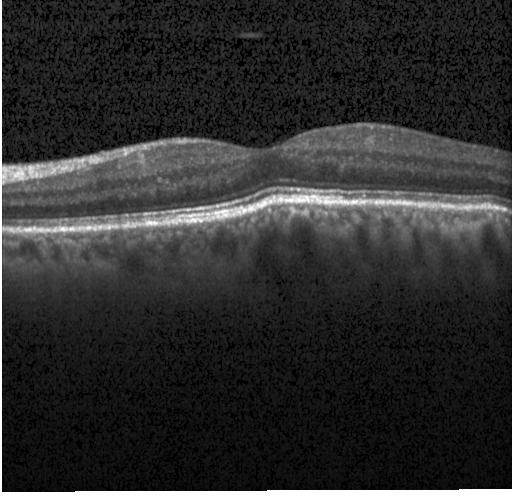

Horizontal scan through the fovea; retinal OCT B-scan
Assessment: no evidence of CNV, DME, or drusen.